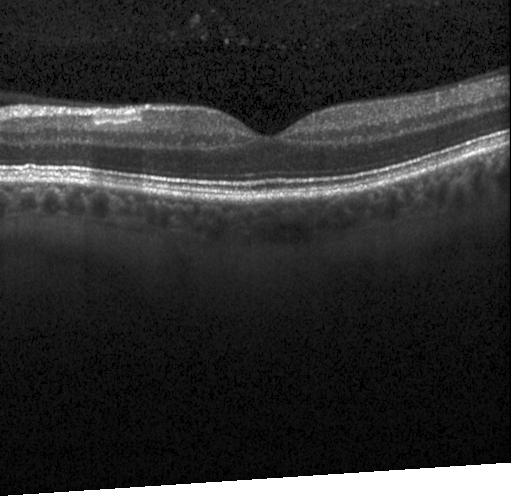 OCT B-scan showing neither choroidal neovascularization, diabetic macular edema, nor drusen.